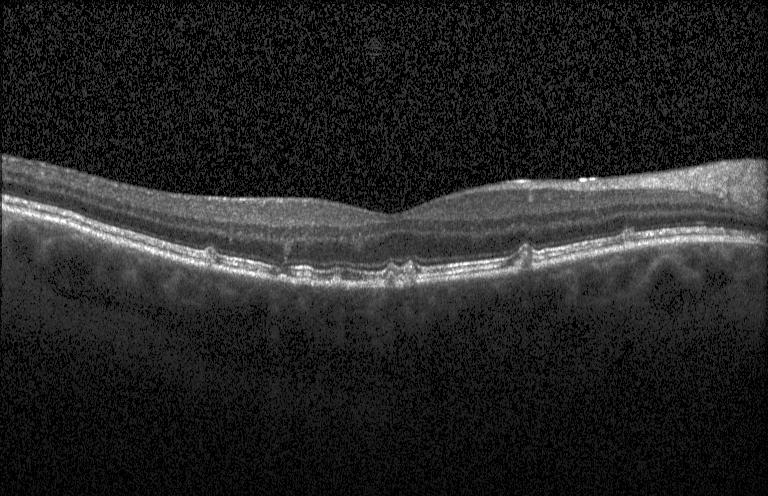

Acquired on a Heidelberg Spectralis, through the macula, spectral-domain optical coherence tomography, optical coherence tomography scan — Finding: multiple drusen.